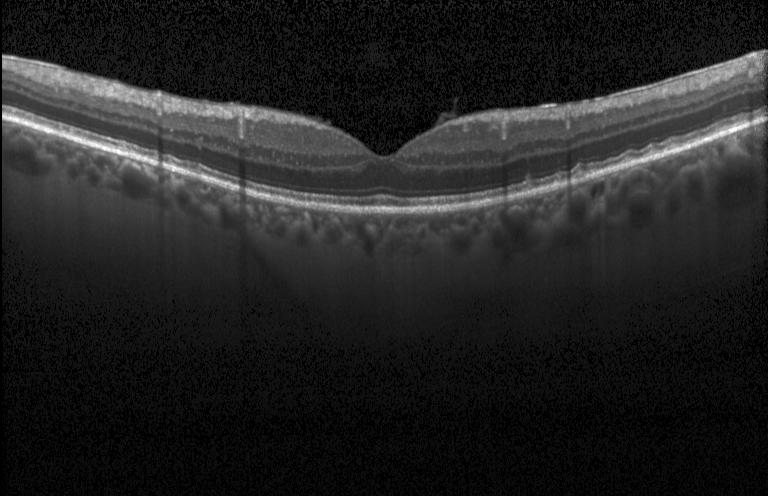 Diagnosis: drusen.